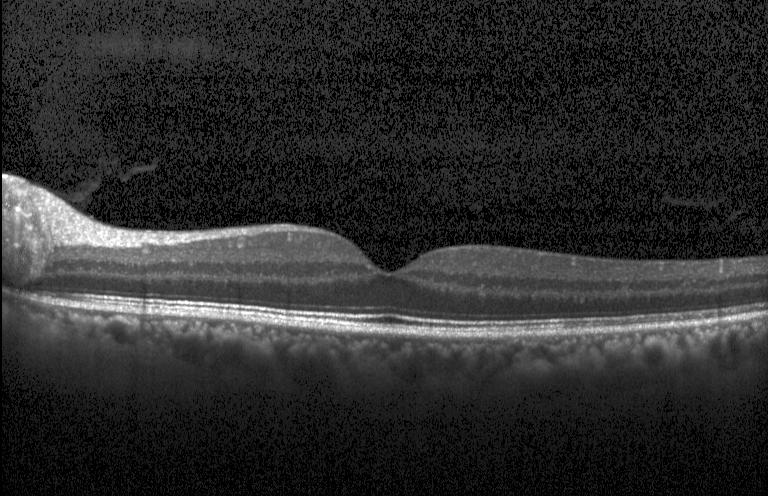 Macular OCT: no choroidal neovascularization, diabetic macular edema, or drusen.